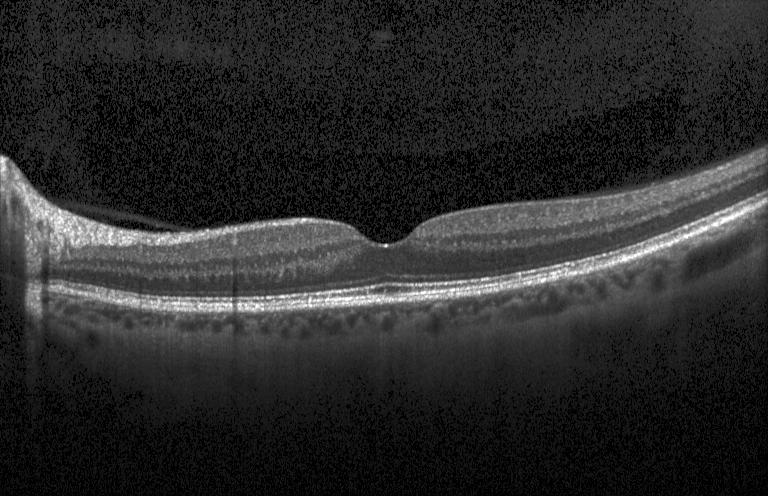 Impression: no choroidal neovascularization, diabetic macular edema, or drusen.